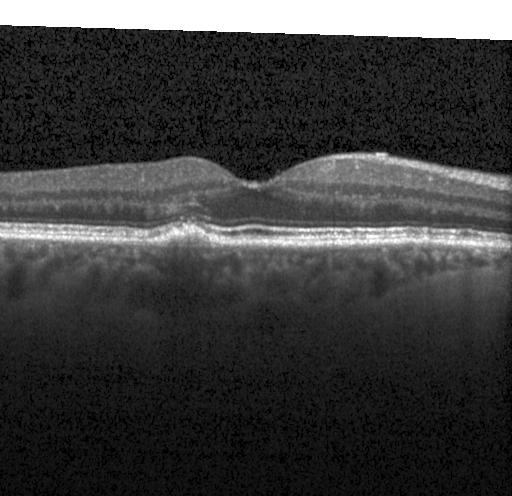
Assessment: drusen.